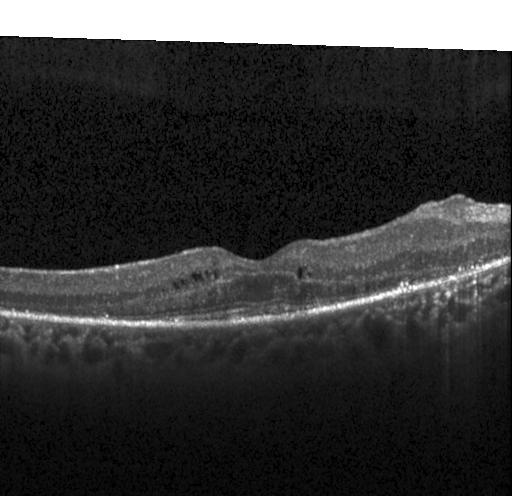 Optical coherence tomography scan. Acquired on a Heidelberg Spectralis. Spectral-domain OCT. Dx: DME.